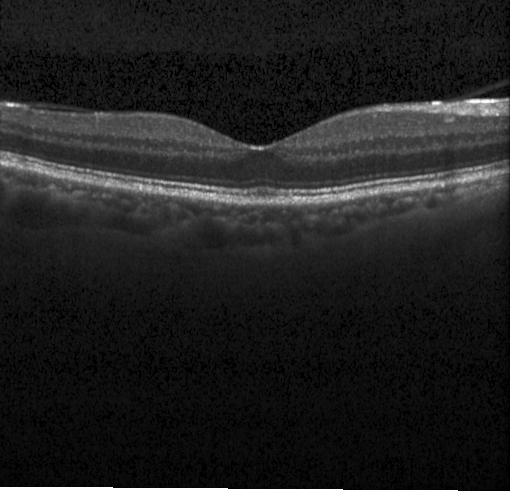 Retinal OCT cross-section showing no evidence of choroidal neovascularization, diabetic macular edema, or drusen.